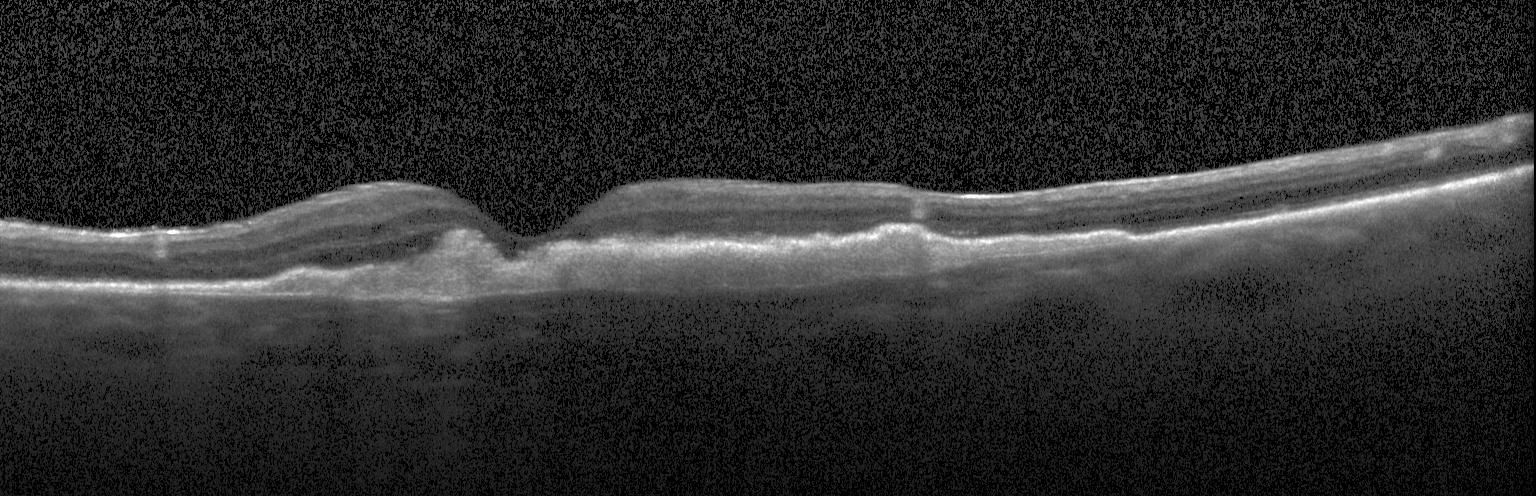

OCT line scan; instrument: Heidelberg Spectralis.
A choroidal neovascular membrane.